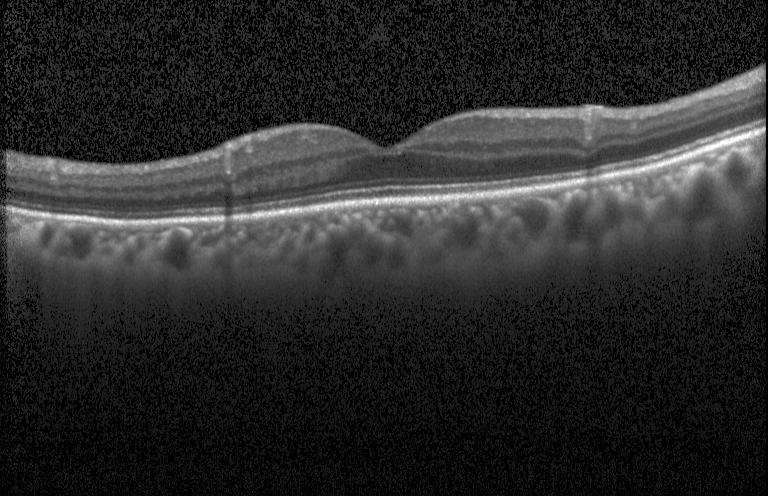
Retinal OCT cross-section
Finding: no choroidal neovascularization, diabetic macular edema, or drusen.